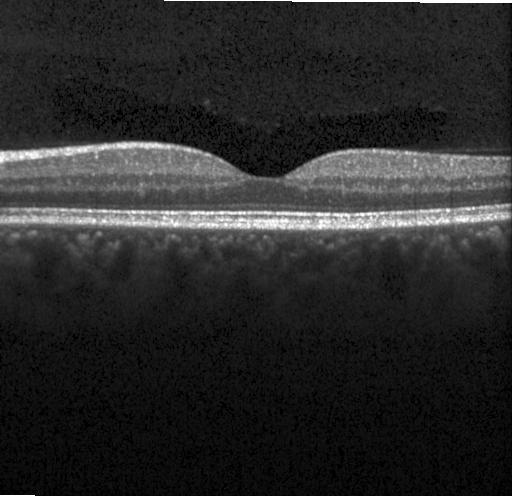
Optical coherence tomography B-scan — Finding: no evidence of choroidal neovascularization, diabetic macular edema, or drusen.